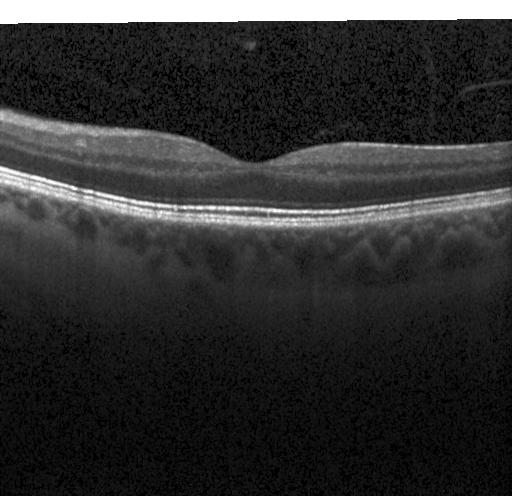

Optical coherence tomography scan. SD-OCT. Neither choroidal neovascularization, diabetic macular edema, nor drusen.